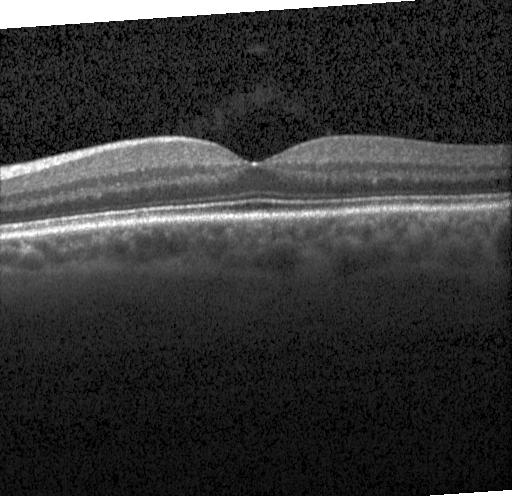

Macular OCT: no CNV, no DME, and no drusen.